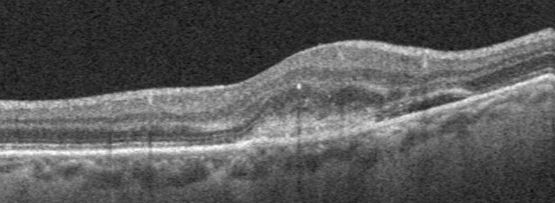 Diagnosis: age-related macular degeneration.